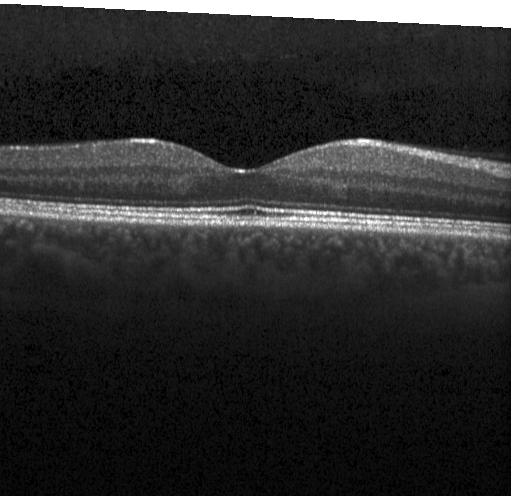
Spectral-domain optical coherence tomography · through the macula · acquired on a Heidelberg Spectralis · OCT line scan
This B-scan demonstrates neither CNV, DME, nor drusen.